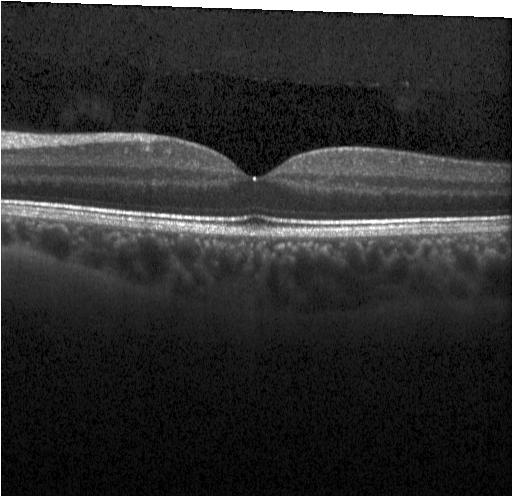 Centered on the fovea, OCT line scan.
This B-scan demonstrates no evidence of choroidal neovascularization, diabetic macular edema, or drusen.